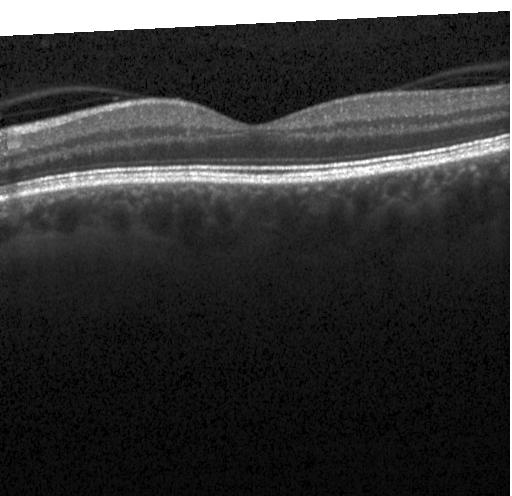

Retinal OCT B-scan
Finding: neither choroidal neovascularization, diabetic macular edema, nor drusen.